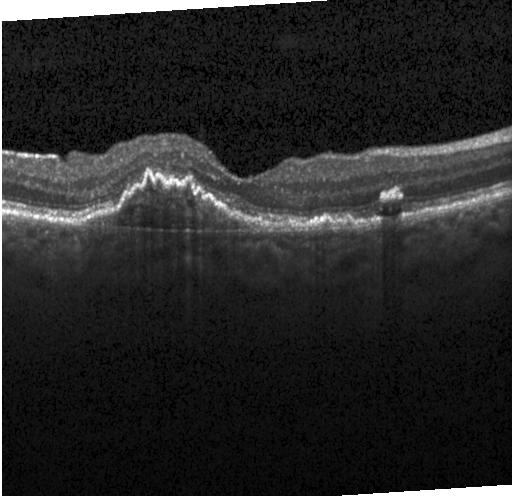

OCT B-scan
Diagnosis: a choroidal neovascular membrane.